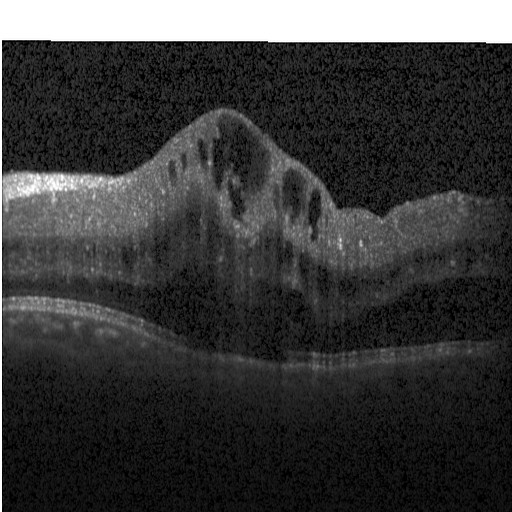 DME.